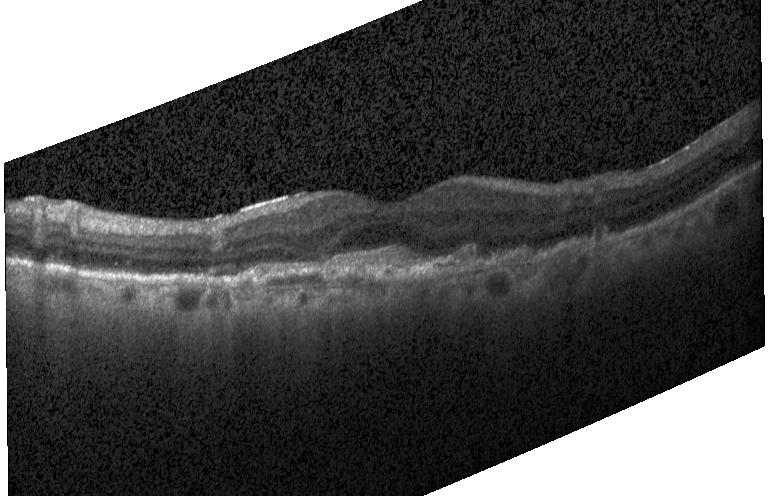 OCT finding: CNV.